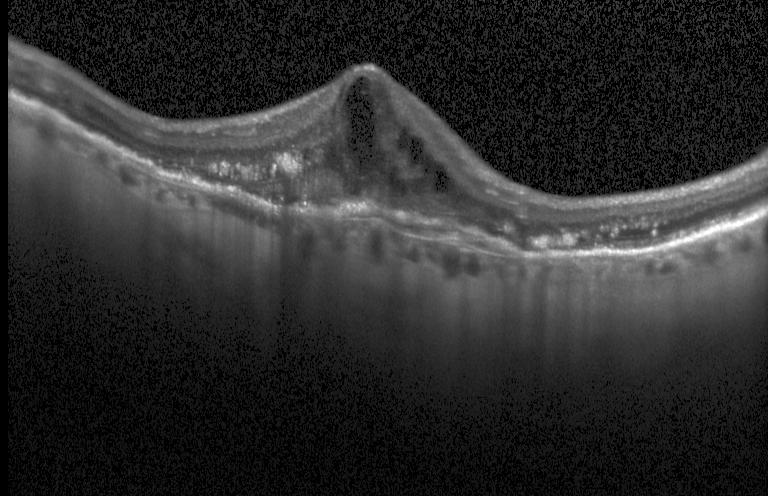
Macular OCT demonstrating choroidal neovascularization.